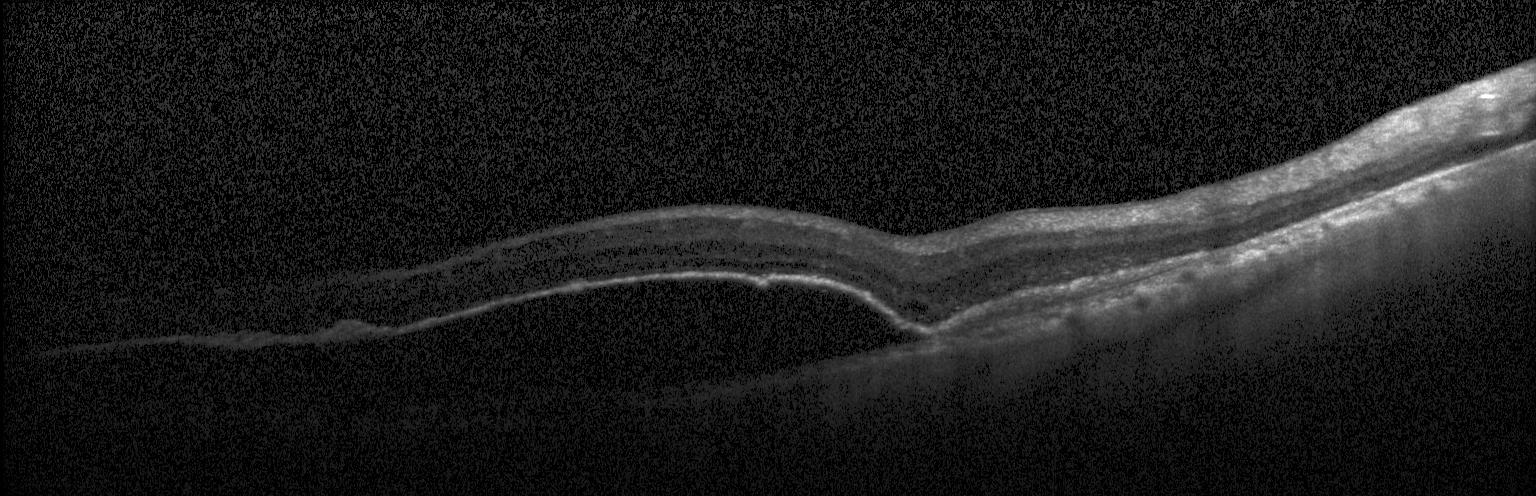

OCT scan showing choroidal neovascularization.